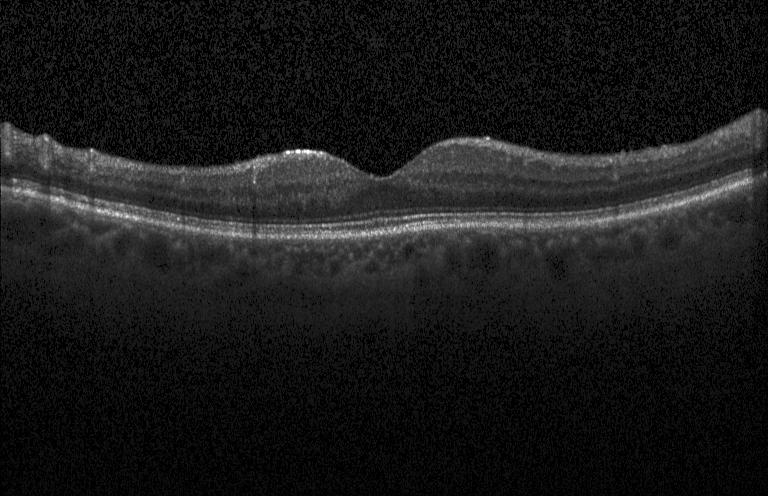
Heidelberg Spectralis, macular scan, OCT line scan — Diagnosis: no evidence of CNV, DME, or drusen.